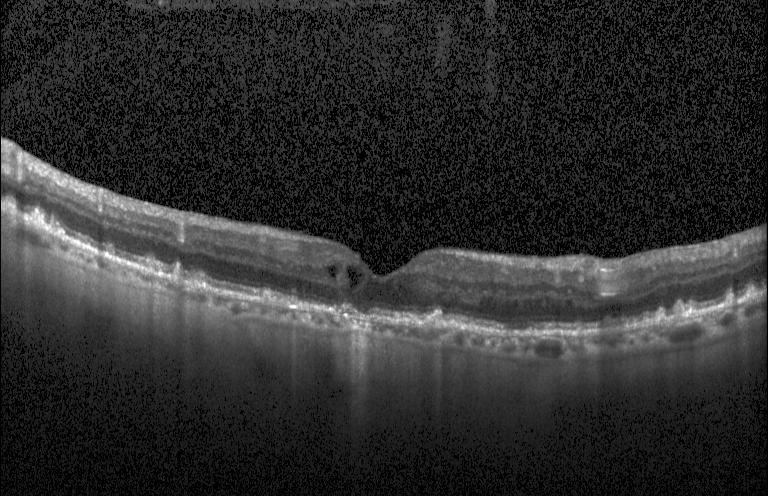

Centered on the fovea; SD-OCT; OCT line scan
The scan shows CNV.